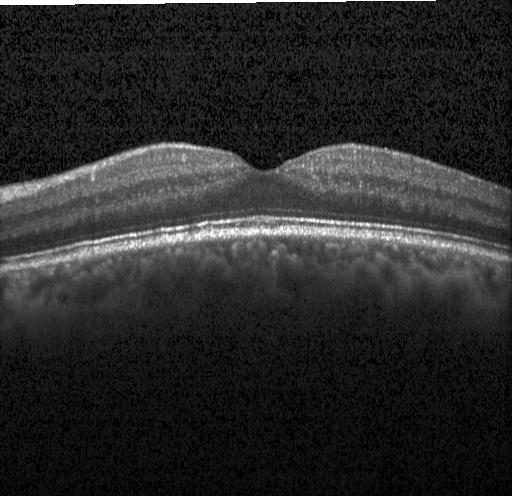
OCT B-scan showing no evidence of choroidal neovascularization, diabetic macular edema, or drusen.